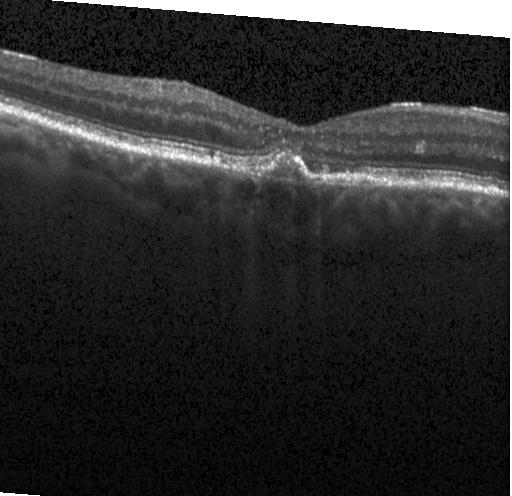
Horizontal scan through the fovea; optical coherence tomography scan.
This B-scan demonstrates choroidal neovascularization (CNV).